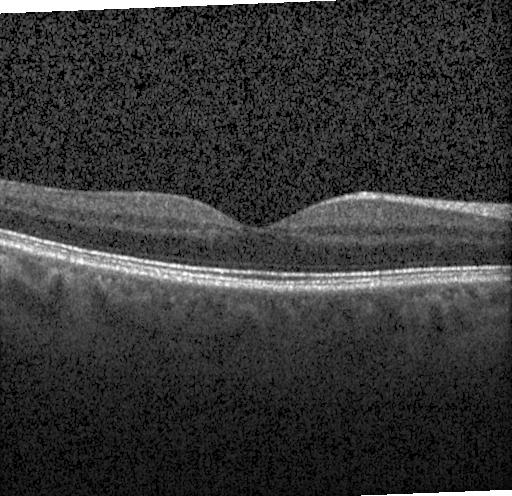

Optical coherence tomography scan · spectral-domain optical coherence tomography — Assessment: no choroidal neovascularization, no diabetic macular edema, and no drusen.